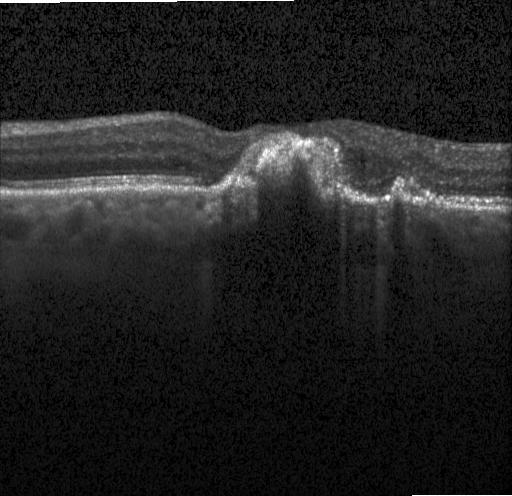 OCT B-scan. Spectral-domain OCT. Centered on the fovea
Dx: choroidal neovascularization.